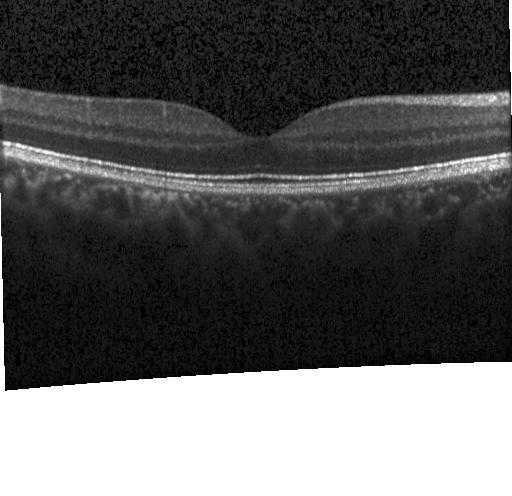 Optical coherence tomography B-scan.
Diagnosis: neither choroidal neovascularization, diabetic macular edema, nor drusen.